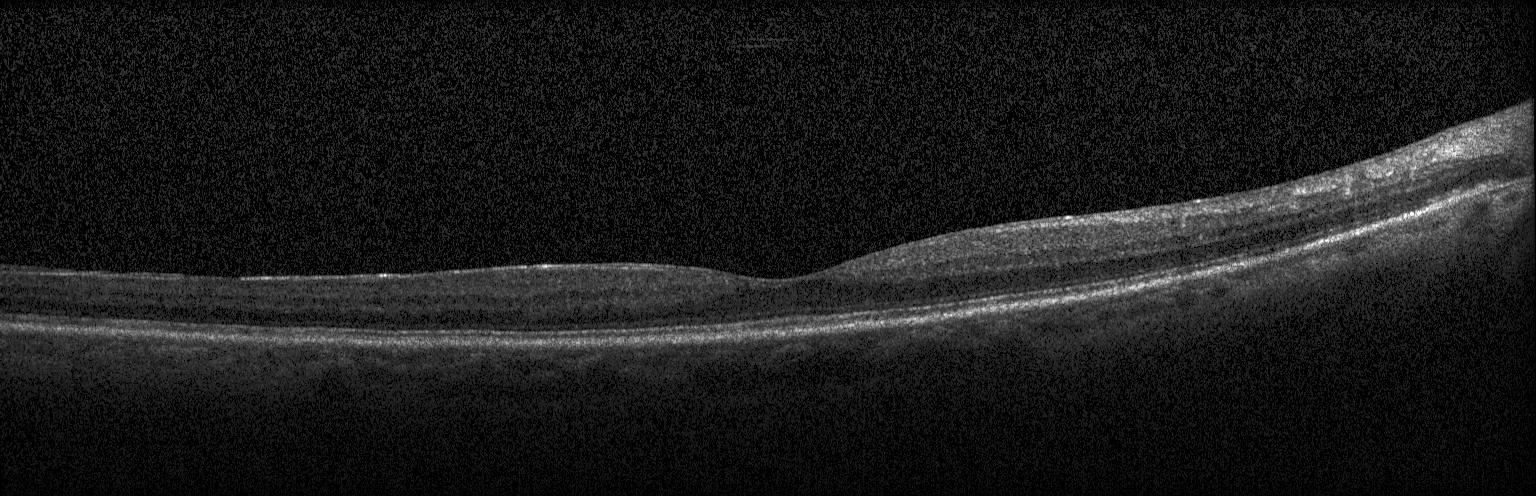

Optical coherence tomography scan. Assessment: no evidence of choroidal neovascularization, diabetic macular edema, or drusen.